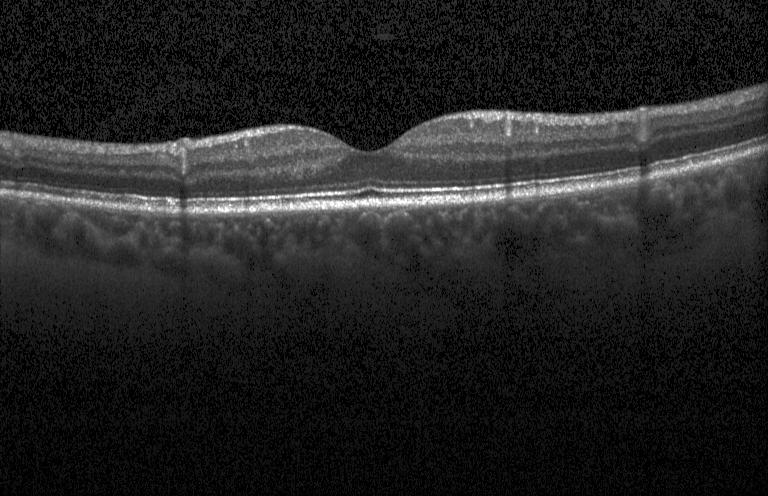

Retinal OCT B-scan · spectral-domain OCT — Diagnosis: no choroidal neovascularization, diabetic macular edema, or drusen.